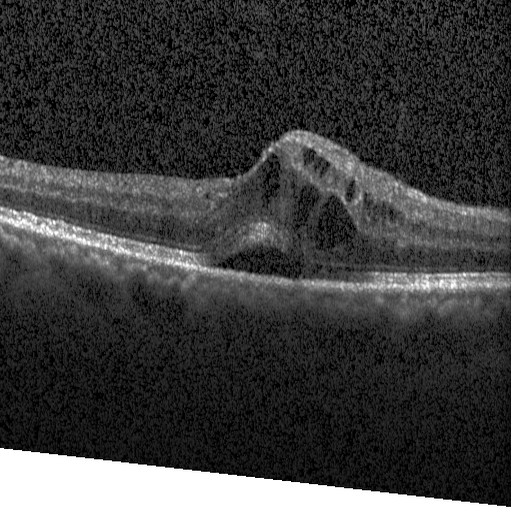
Finding: DME.